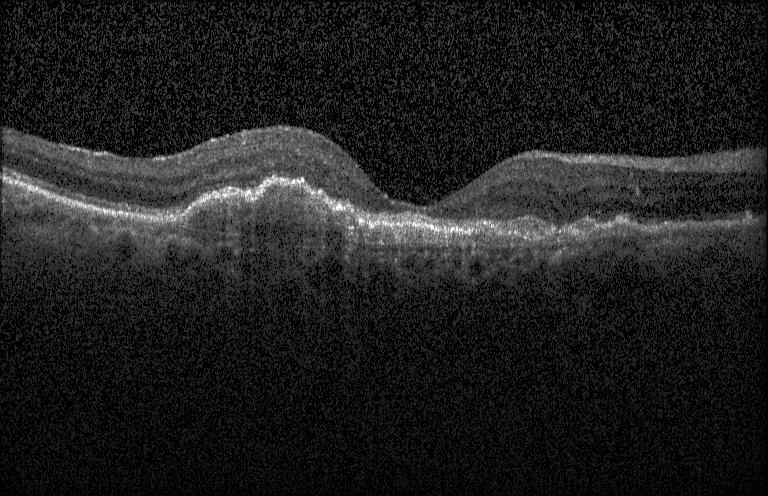
Assessment: choroidal neovascularization (CNV).